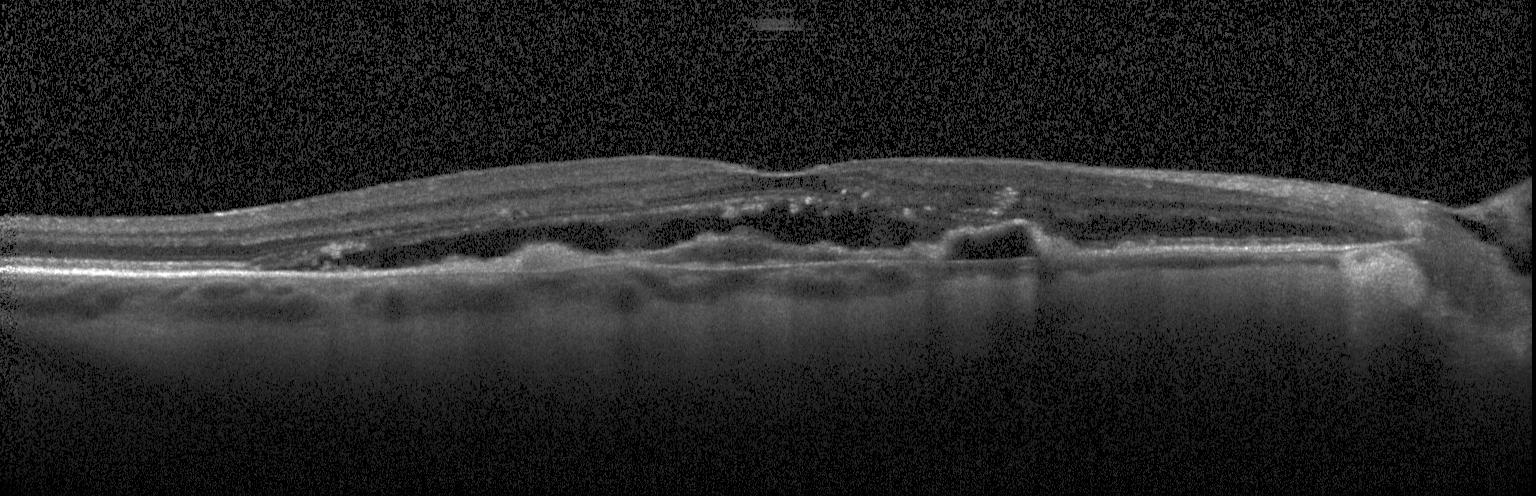

OCT line scan. Spectral-domain OCT. Horizontal scan through the fovea. Heidelberg Spectralis OCT system. Finding: a choroidal neovascular membrane.